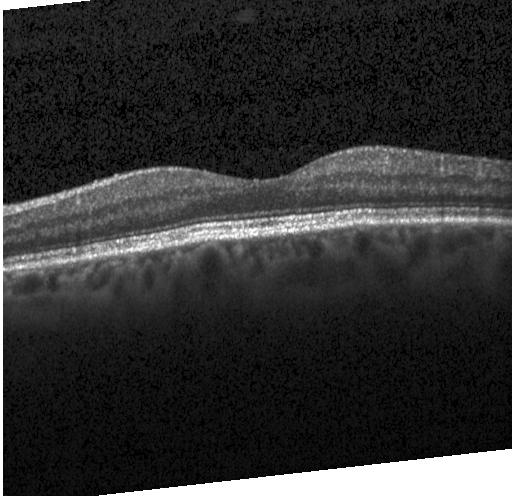 Optical coherence tomography scan.
Impression: no CNV, DME, or drusen.